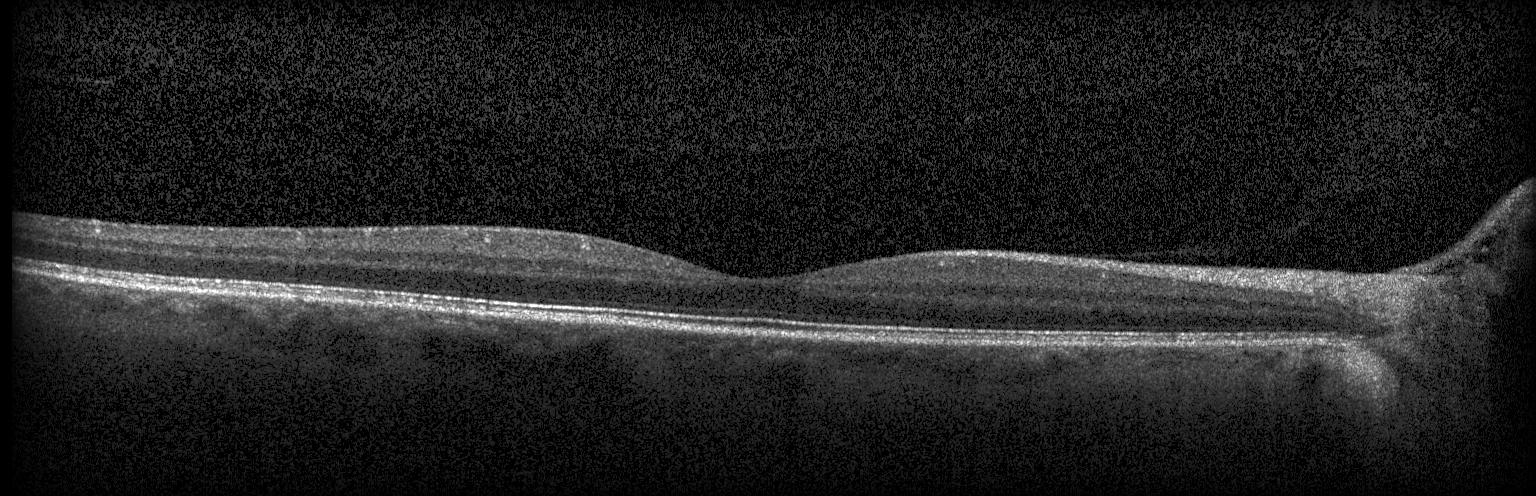

OCT B-scan · centered on the fovea. Neither choroidal neovascularization, diabetic macular edema, nor drusen.